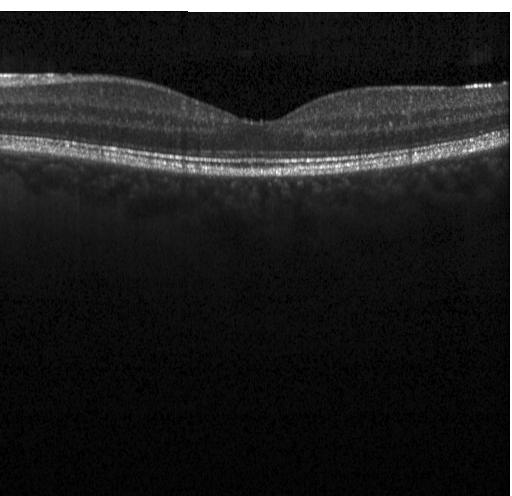 Heidelberg Spectralis OCT system. Through the macula. Retinal OCT B-scan
OCT finding: no CNV, no DME, and no drusen.